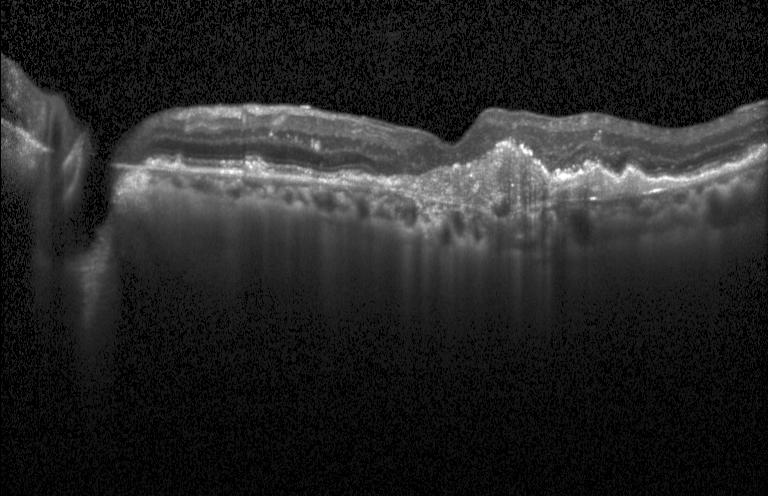 OCT line scan
Macular OCT: choroidal neovascularization (CNV).